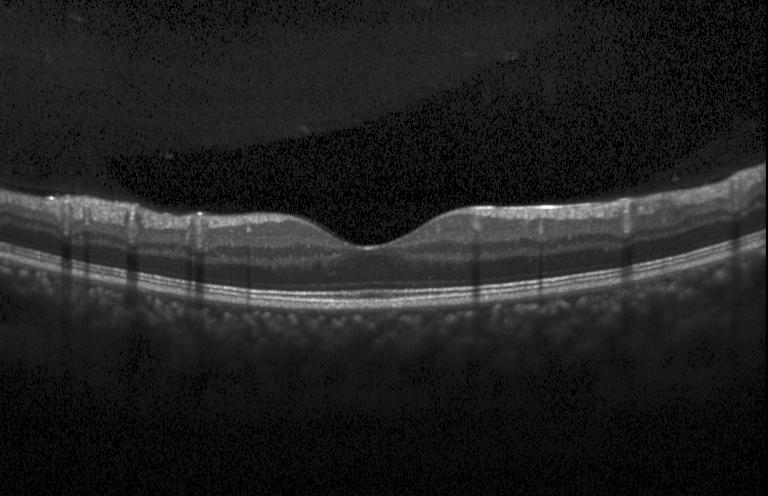
Impression: no CNV, DME, or drusen.